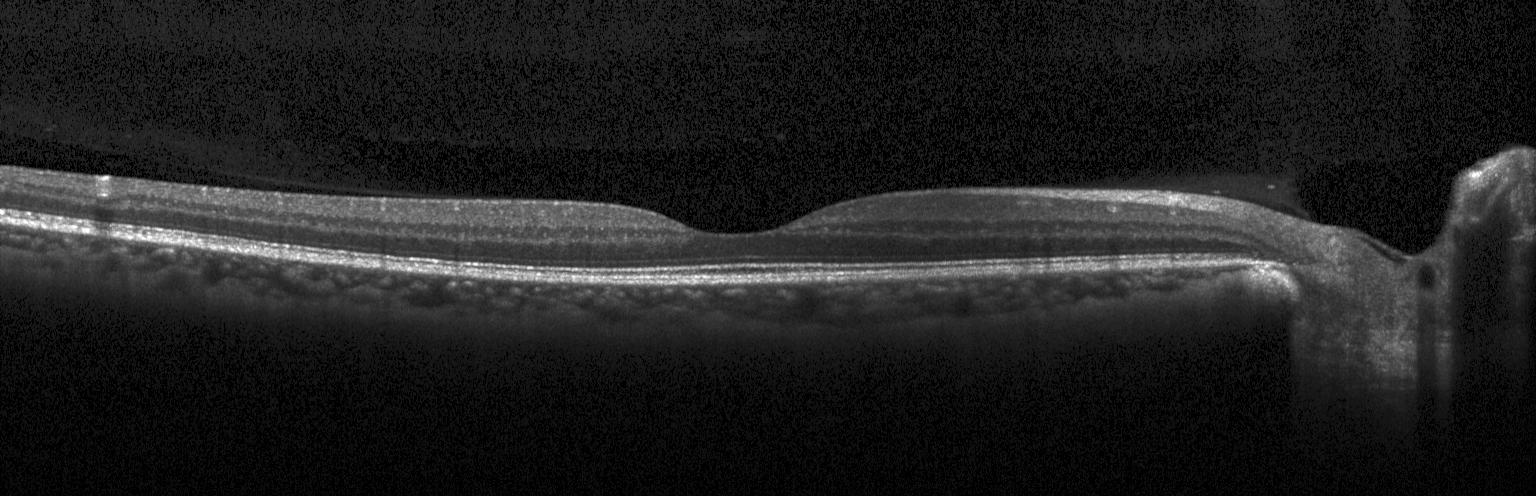

OCT B-scan, SD-OCT — Diagnosis: no choroidal neovascularization, diabetic macular edema, or drusen.